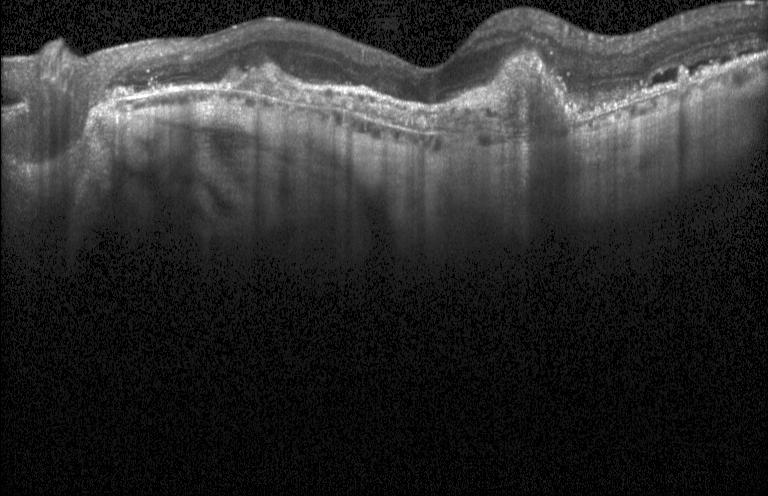 OCT B-scan, fovea-centered, SD-OCT, instrument: Heidelberg Spectralis — Impression: choroidal neovascularization.